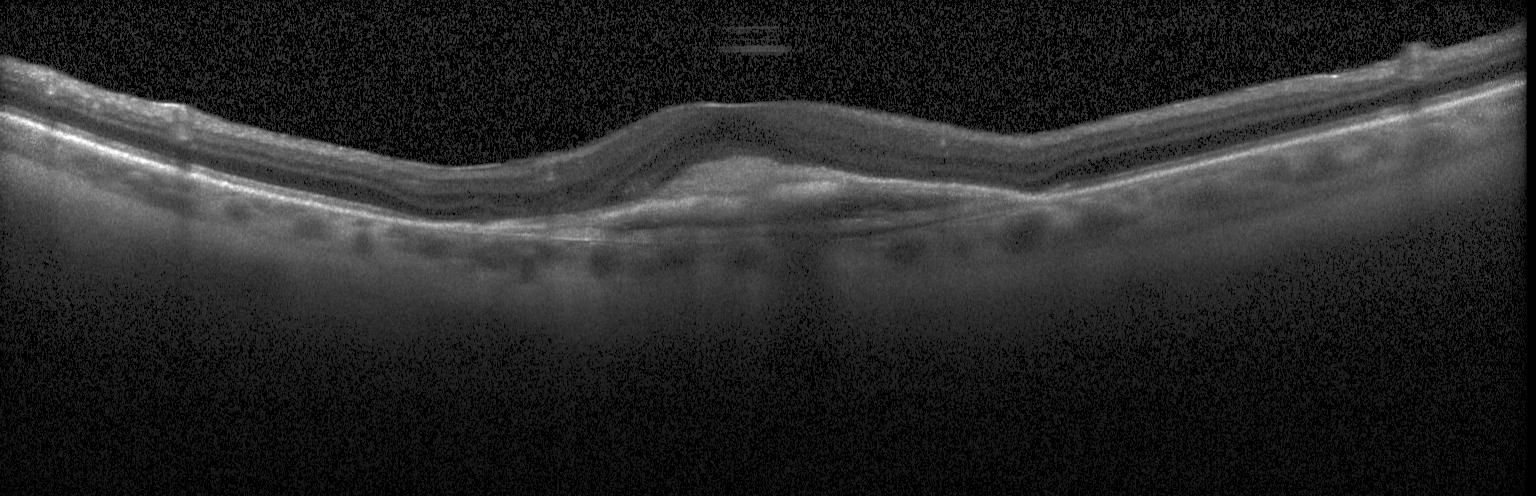
Diagnosis: choroidal neovascularization (CNV).